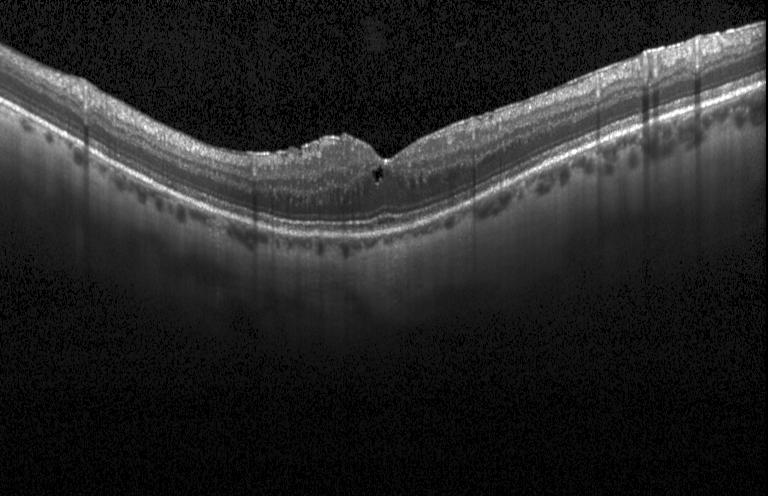

Finding: diabetic macular edema.